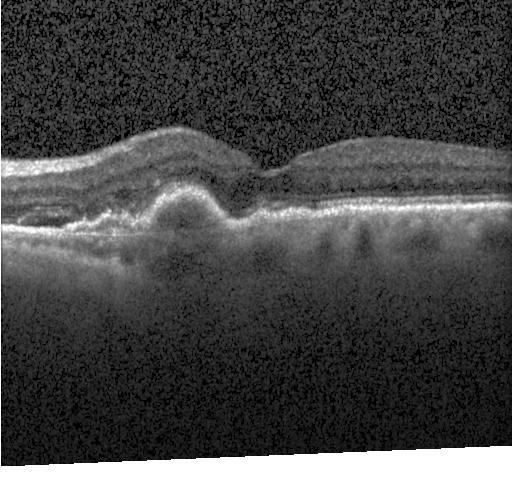
Diagnosis: a choroidal neovascular membrane.